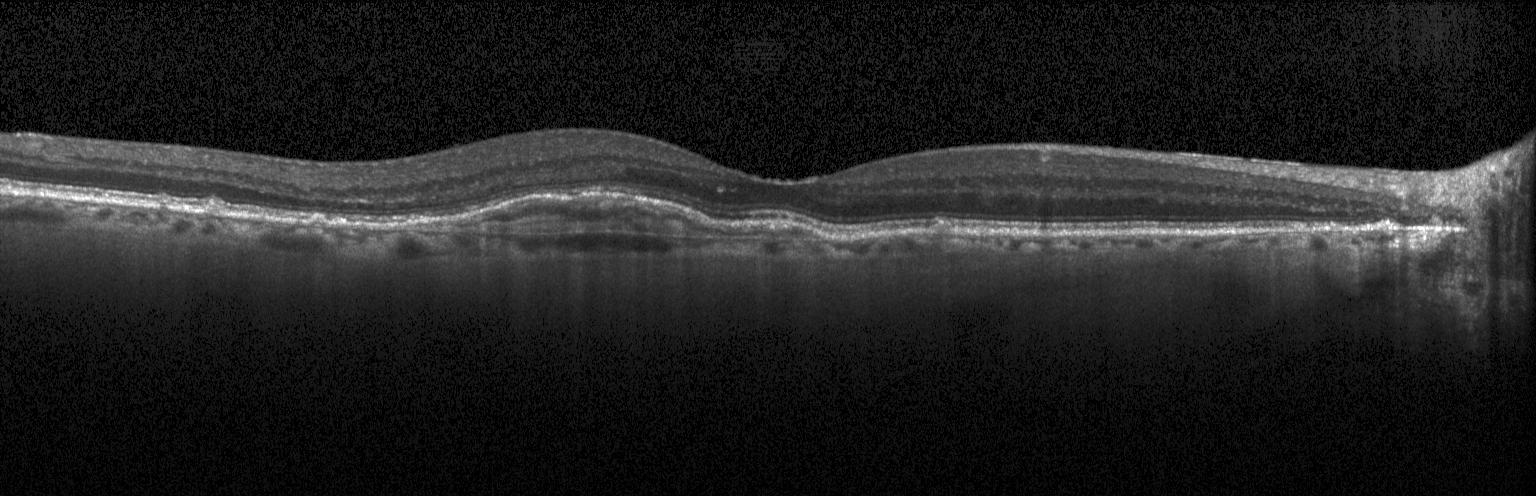

Optical coherence tomography B-scan, instrument: Heidelberg Spectralis
Finding: CNV.